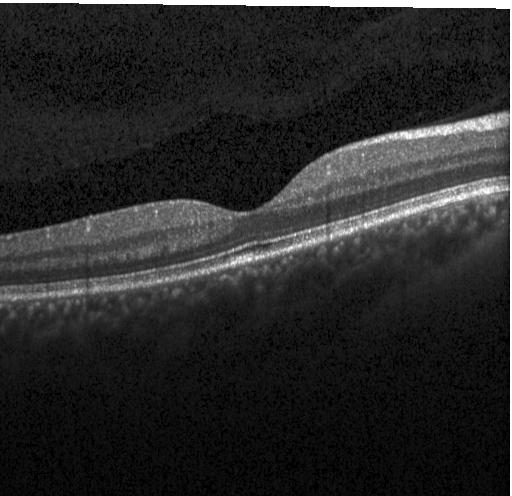 SD-OCT. Optical coherence tomography B-scan. Macular scan.
Diagnosis: no choroidal neovascularization, diabetic macular edema, or drusen.